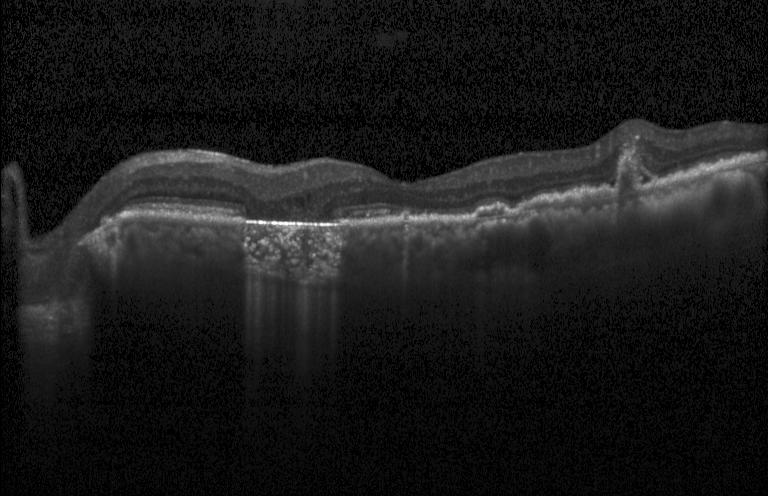
Optical coherence tomography scan; Heidelberg Spectralis OCT system; spectral-domain optical coherence tomography — The scan shows choroidal neovascularization (CNV).